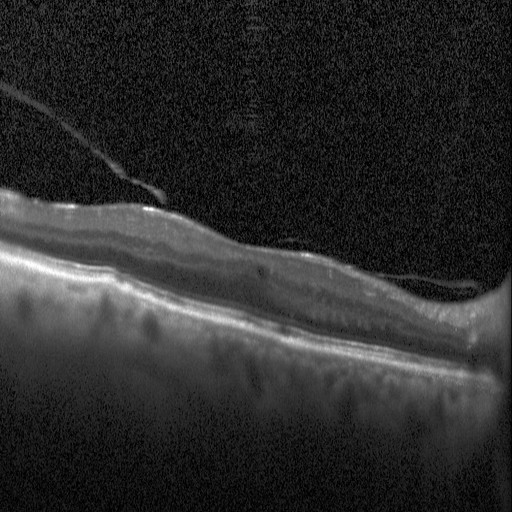

Dx: DME.